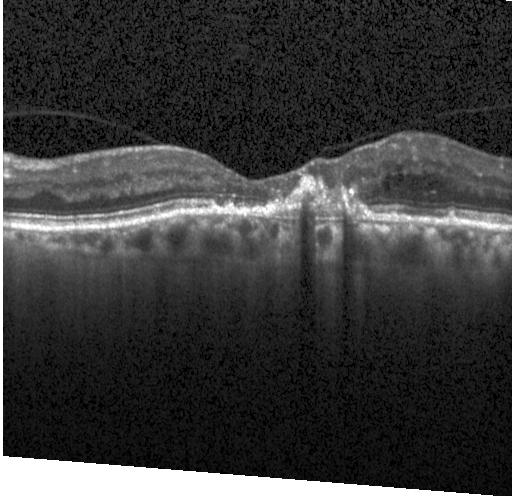

Spectral-domain OCT B-scan: CNV.